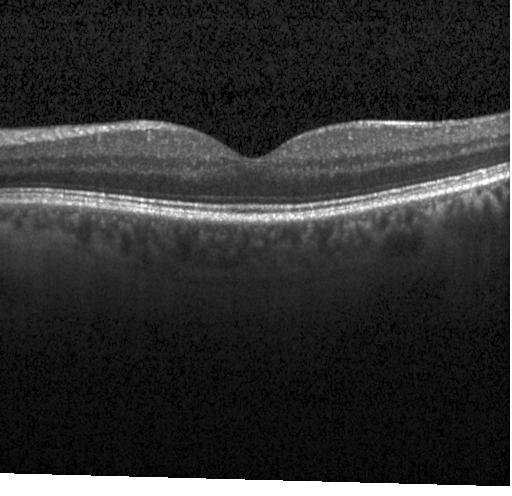

Spectral-domain optical coherence tomography; centered on the fovea; optical coherence tomography B-scan; acquired on a Heidelberg Spectralis. Impression: no evidence of choroidal neovascularization, diabetic macular edema, or drusen.